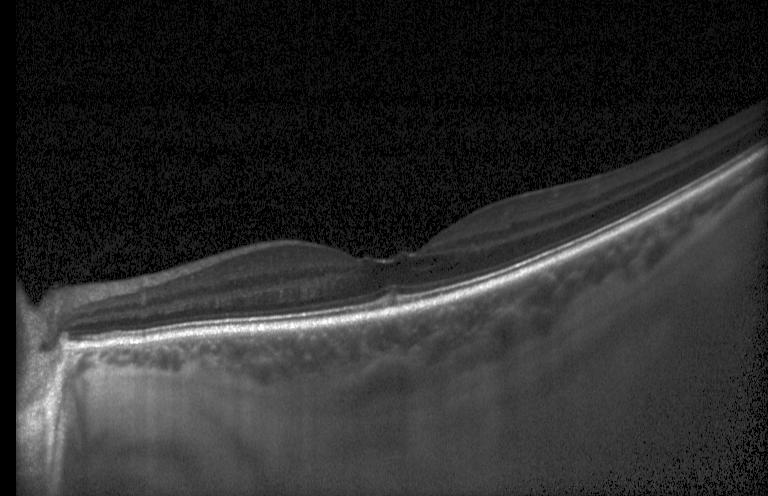 Optical coherence tomography scan. Through the macula. Instrument: Heidelberg Spectralis
Finding: no evidence of CNV, DME, or drusen.